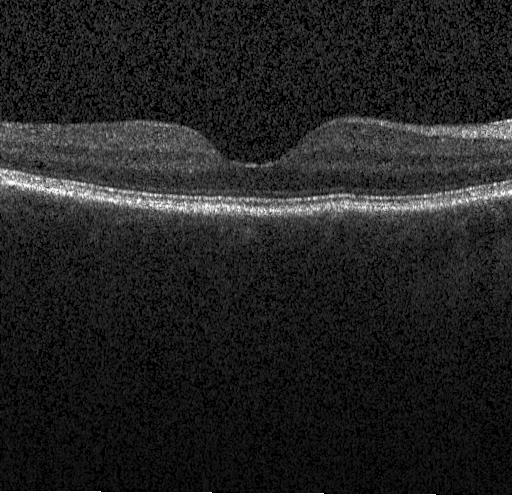

Fovea-centered; retinal OCT cross-section; Heidelberg Spectralis OCT system. Finding: no evidence of choroidal neovascularization, diabetic macular edema, or drusen.